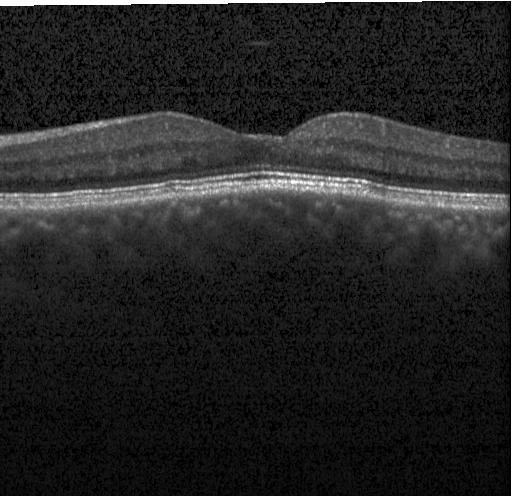 The scan shows neither CNV, DME, nor drusen.